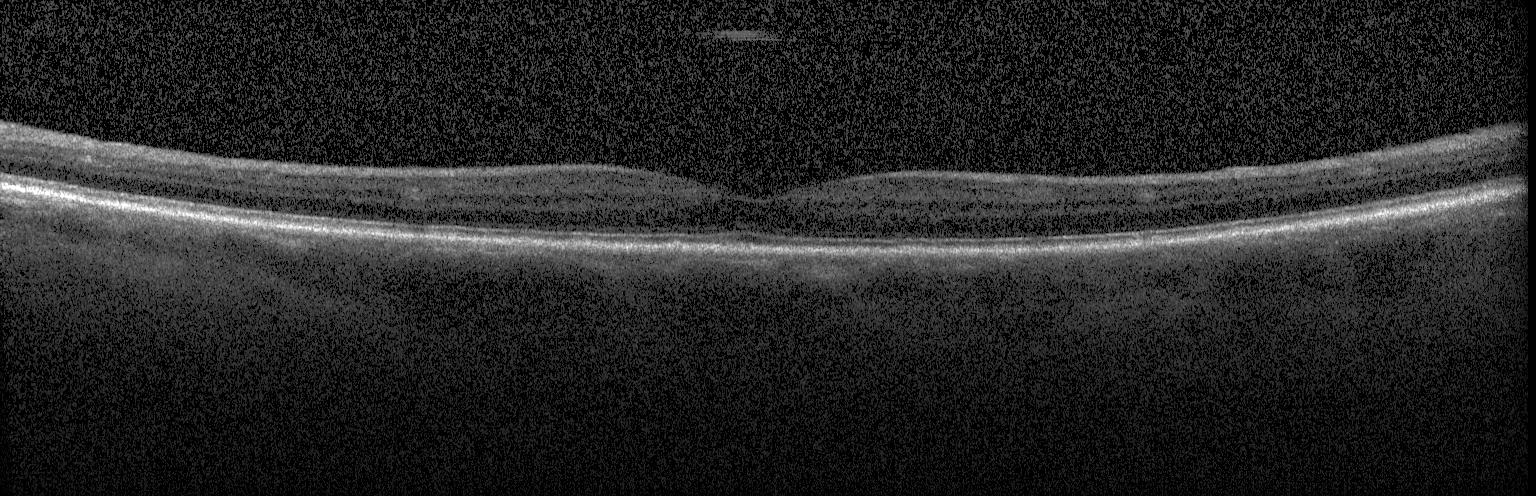 OCT finding: no evidence of CNV, DME, or drusen.